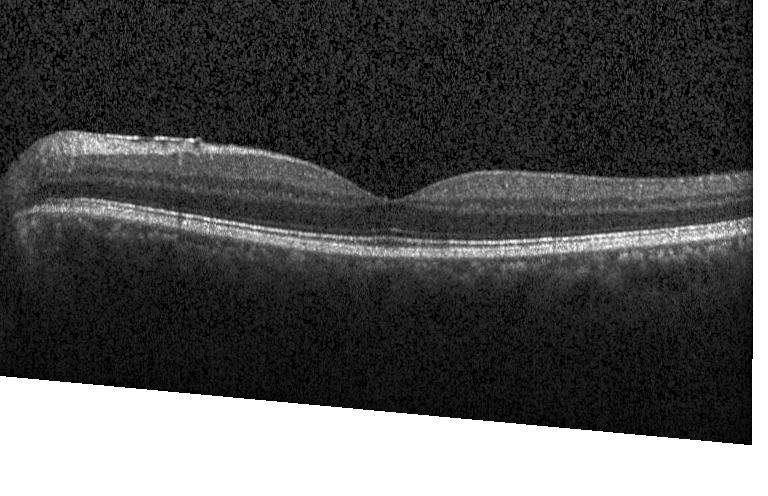
No evidence of choroidal neovascularization, diabetic macular edema, or drusen.